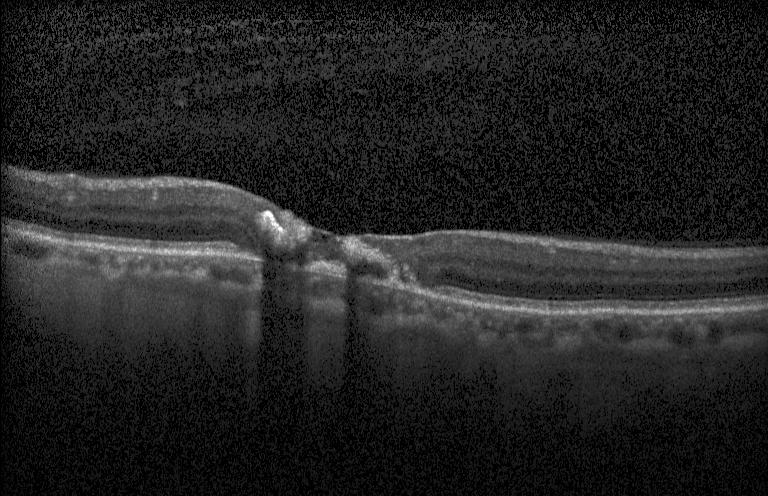
Impression: choroidal neovascularization (CNV).